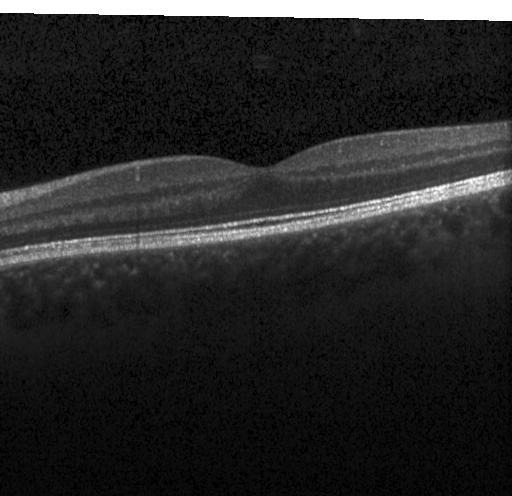

Through the macula. OCT B-scan. Spectral-domain optical coherence tomography. Heidelberg Spectralis OCT system. Macular OCT: no evidence of choroidal neovascularization, diabetic macular edema, or drusen.